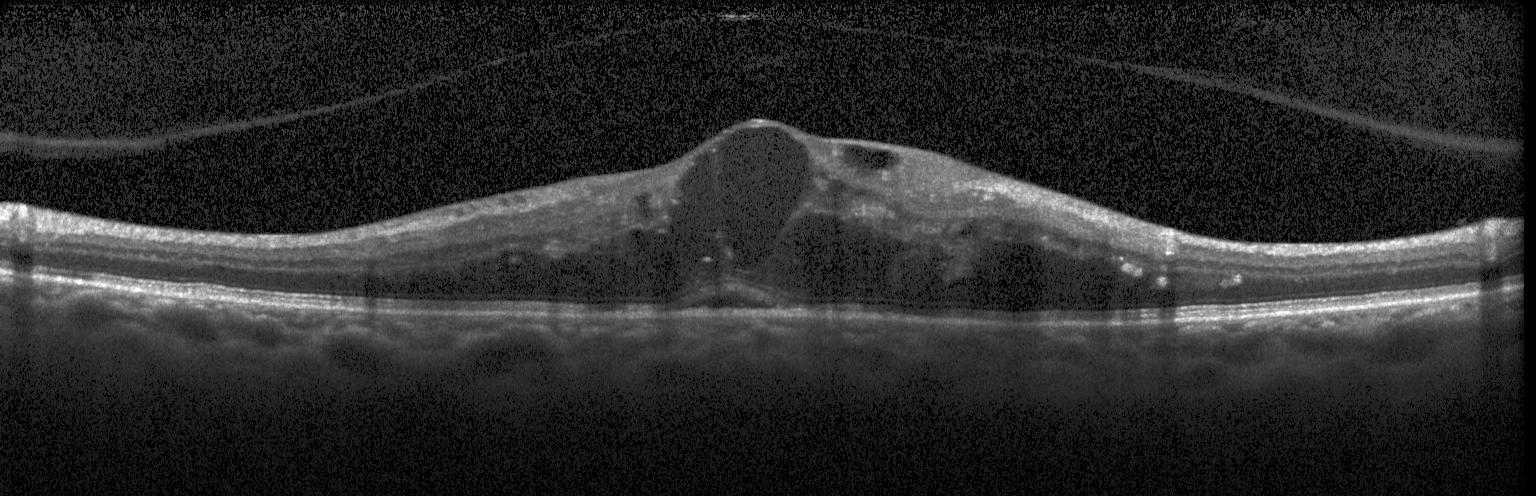
Centered on the fovea, optical coherence tomography scan, SD-OCT — Dx: diabetic macular edema.